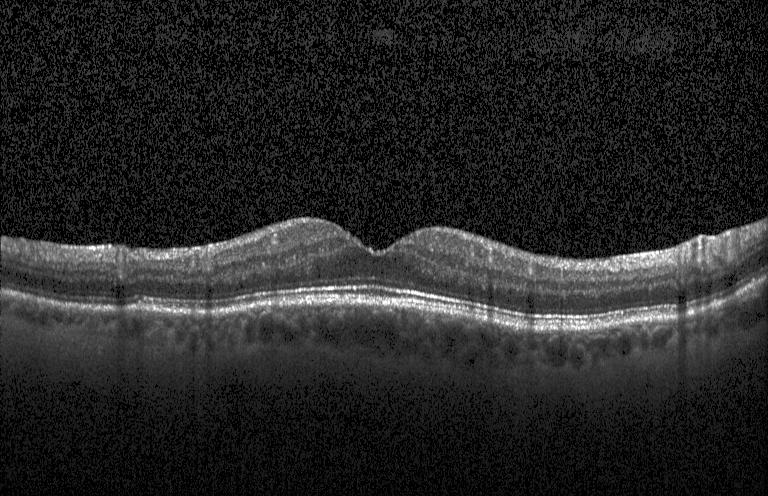

Retinal OCT cross-section showing neither CNV, DME, nor drusen.